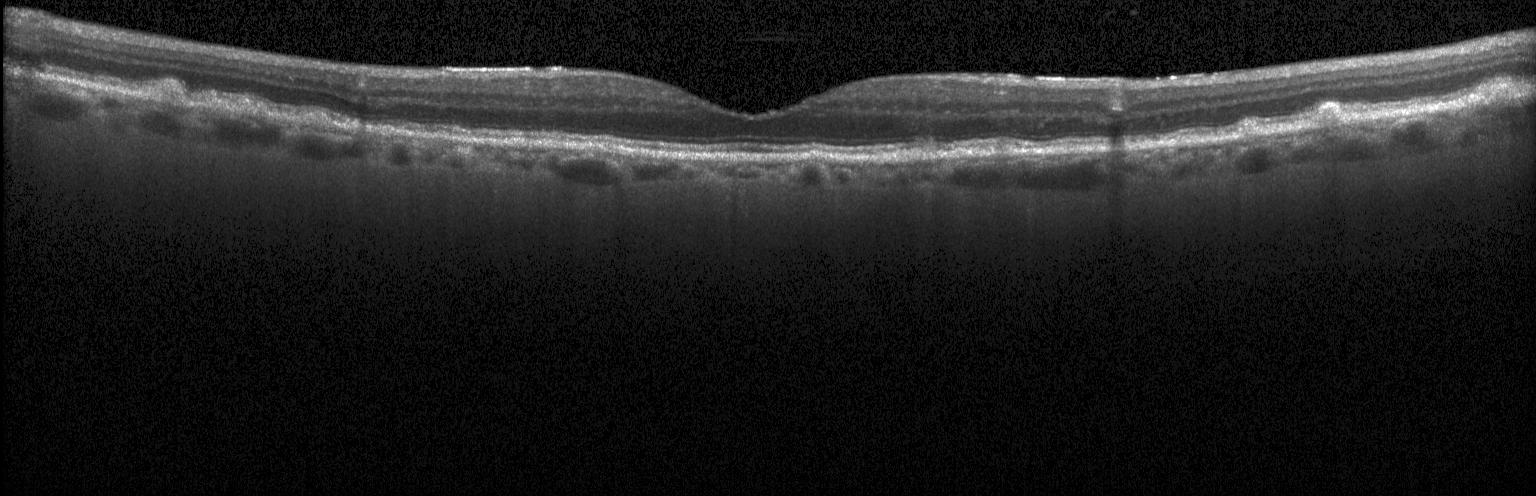

Retinal OCT B-scan
The scan shows multiple drusen.